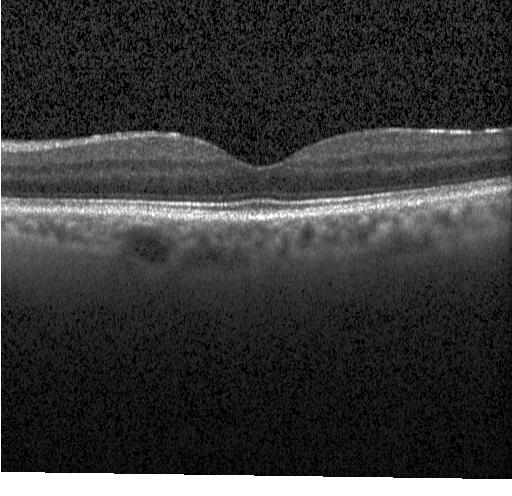
SD-OCT; retinal OCT cross-section.
Finding: no evidence of choroidal neovascularization, diabetic macular edema, or drusen.